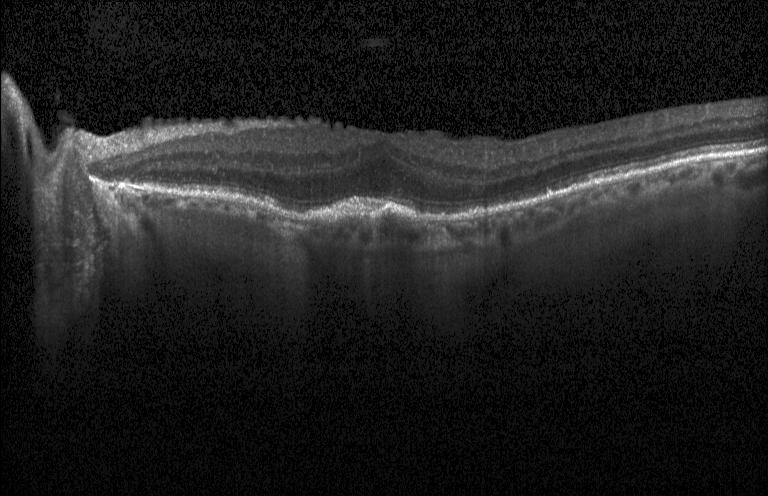 Macular scan; optical coherence tomography B-scan — Impression: choroidal neovascularization.